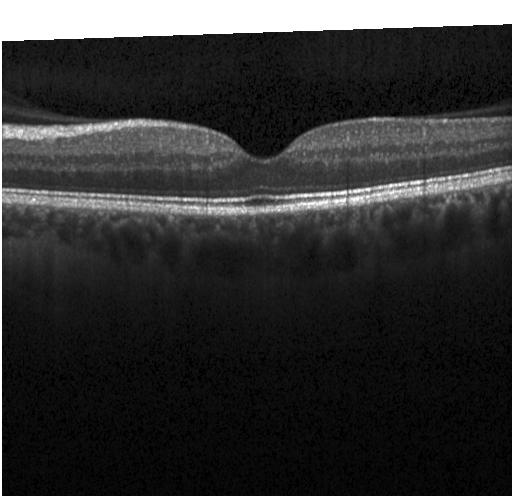
Impression: neither CNV, DME, nor drusen.